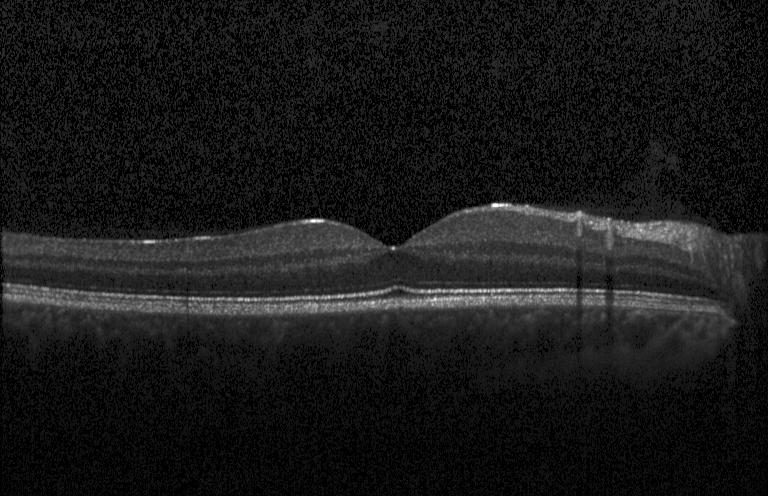
Assessment: neither choroidal neovascularization, diabetic macular edema, nor drusen.